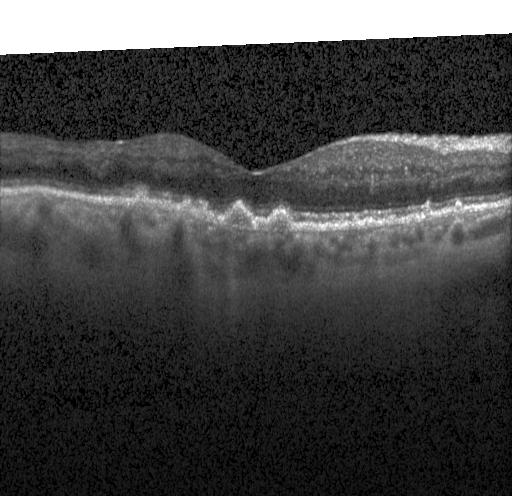

SD-OCT; retinal OCT B-scan
Diagnosis: sub-RPE drusenoid deposits.